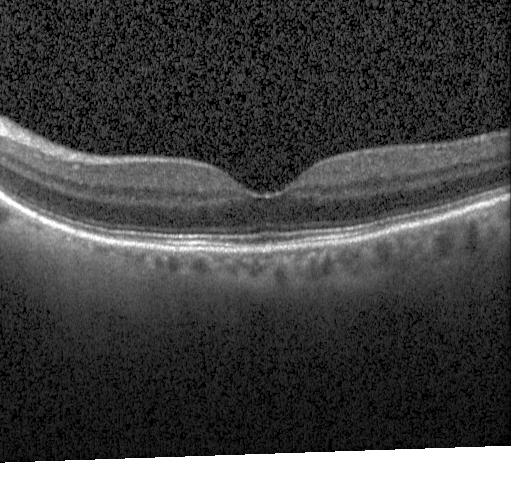
Retinal OCT B-scan; instrument: Heidelberg Spectralis. The scan shows neither choroidal neovascularization, diabetic macular edema, nor drusen.